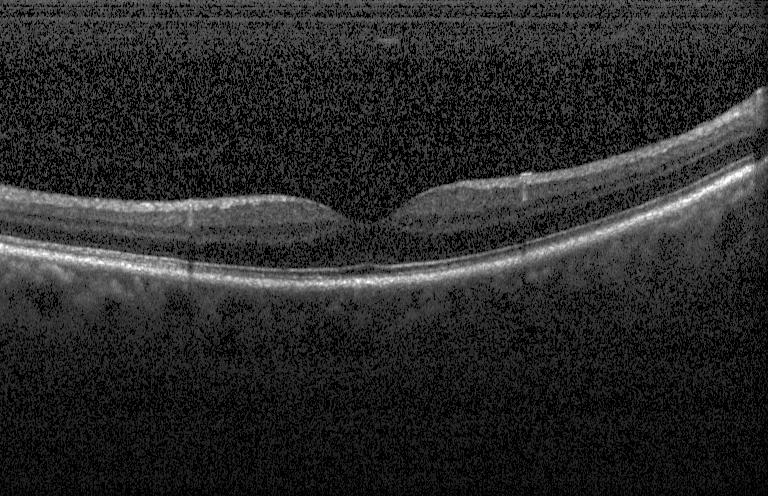

Fovea-centered, Heidelberg Spectralis OCT system, retinal OCT B-scan.
Macular OCT: no choroidal neovascularization, no diabetic macular edema, and no drusen.